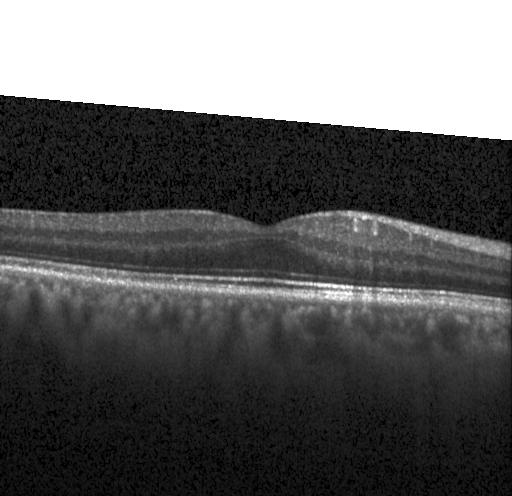 OCT B-scan — Neither choroidal neovascularization, diabetic macular edema, nor drusen.